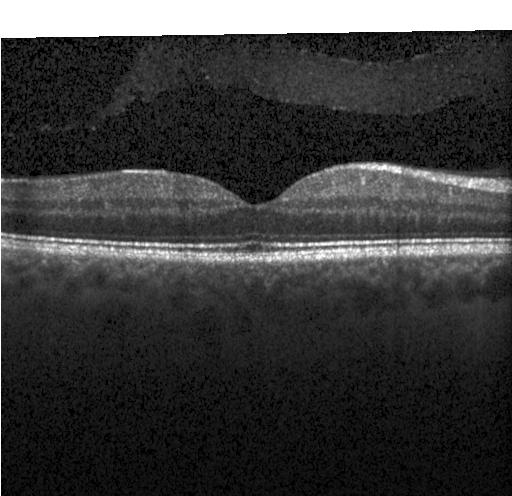 Optical coherence tomography B-scan — This B-scan demonstrates no CNV, DME, or drusen.